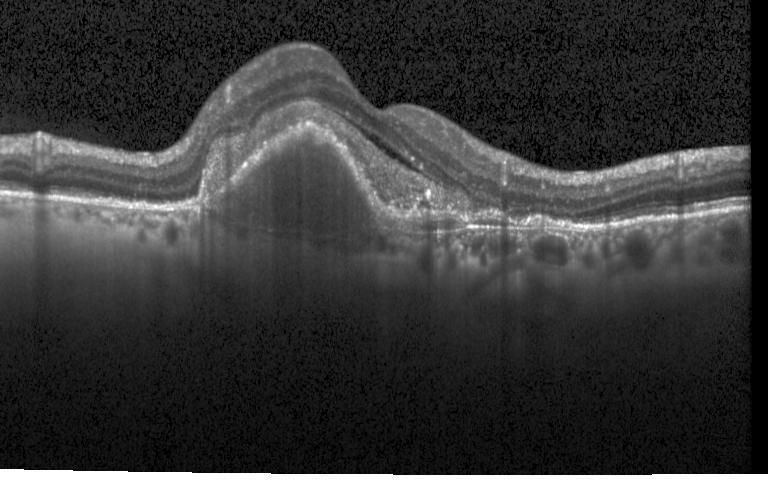
Dx: CNV.